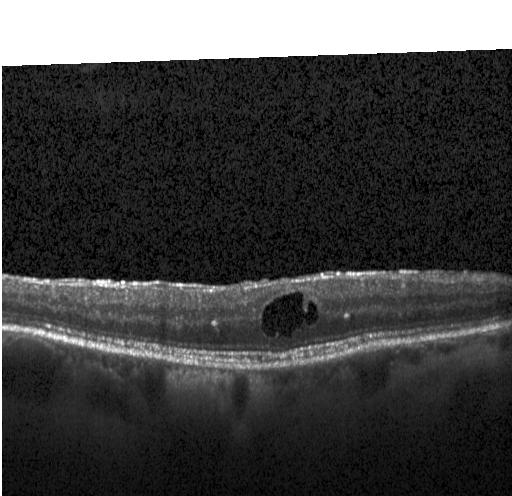 Diabetic macular edema (DME).